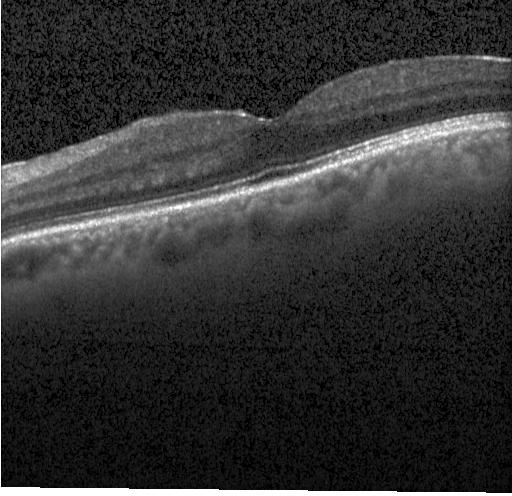

This B-scan demonstrates no evidence of choroidal neovascularization, diabetic macular edema, or drusen.